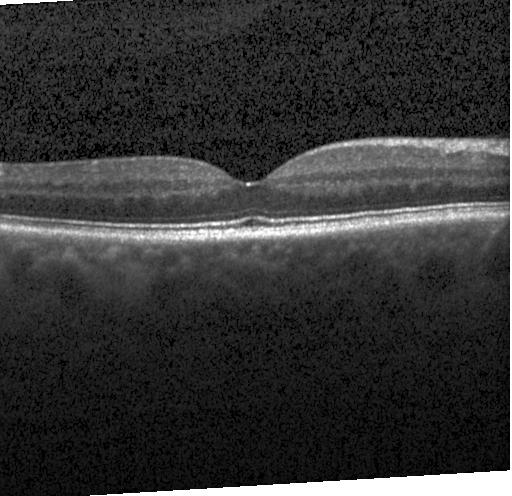
Optical coherence tomography B-scan. Through the macula
Dx: no CNV, DME, or drusen.